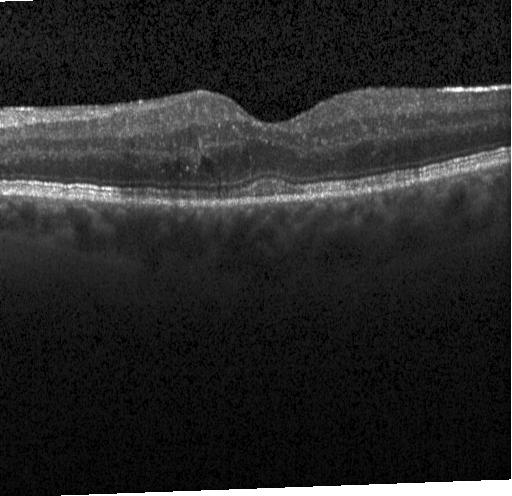

Spectral-domain OCT, OCT B-scan, centered on the fovea, acquired on a Heidelberg Spectralis. OCT finding: diabetic macular edema.